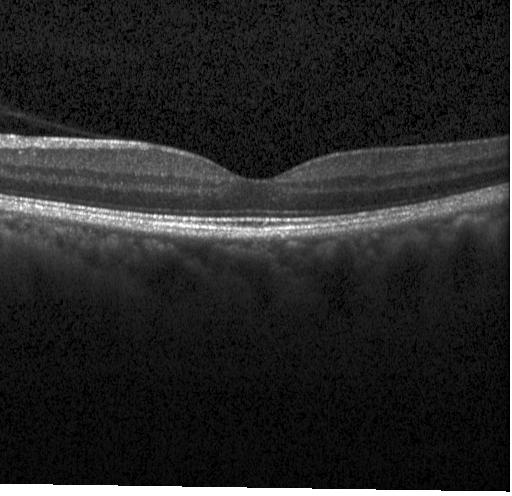
Instrument: Heidelberg Spectralis; fovea-centered; retinal OCT B-scan; SD-OCT.
Diagnosis: no choroidal neovascularization, diabetic macular edema, or drusen.